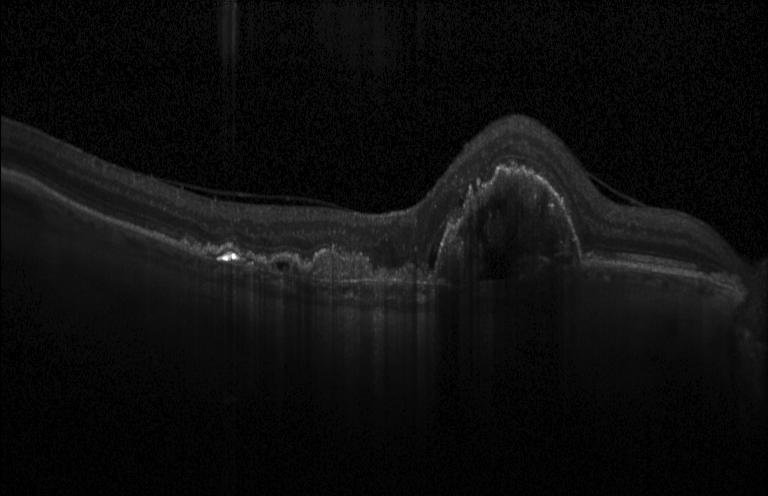
Through the macula, retinal OCT cross-section.
Choroidal neovascularization (CNV).